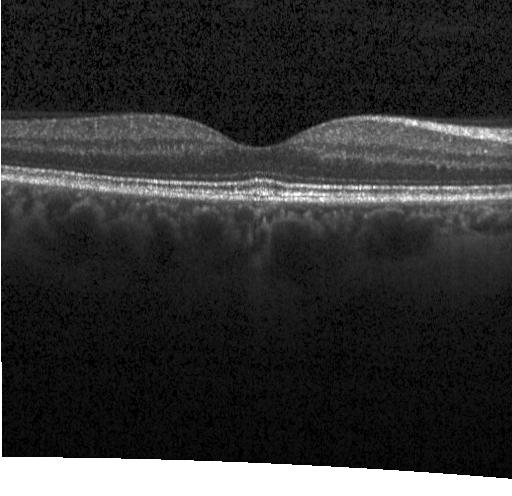

Spectral-domain optical coherence tomography, retinal OCT cross-section, Heidelberg Spectralis OCT system.
This B-scan demonstrates neither CNV, DME, nor drusen.